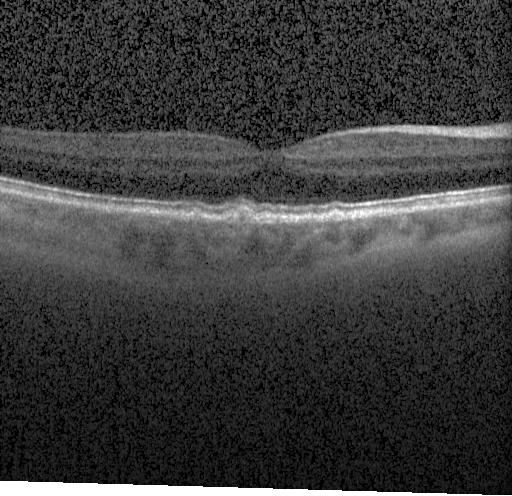 Spectral-domain OCT; Heidelberg Spectralis OCT system; fovea-centered; retinal OCT B-scan. Finding: drusen.